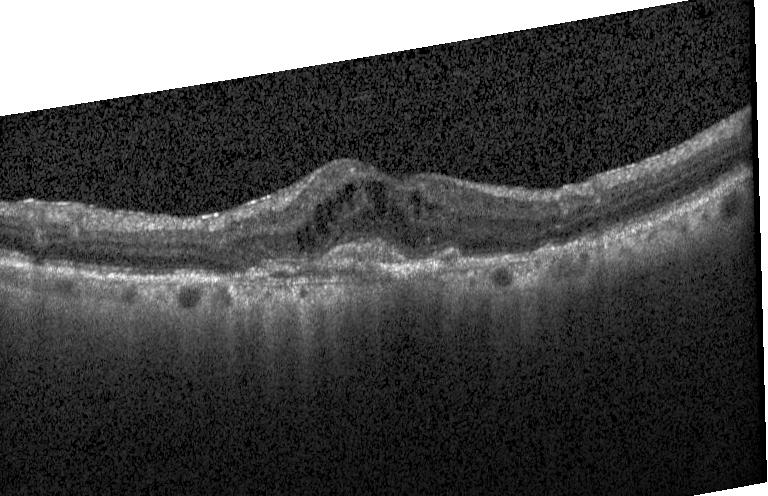 Retinal OCT B-scan. Dx: a choroidal neovascular membrane.